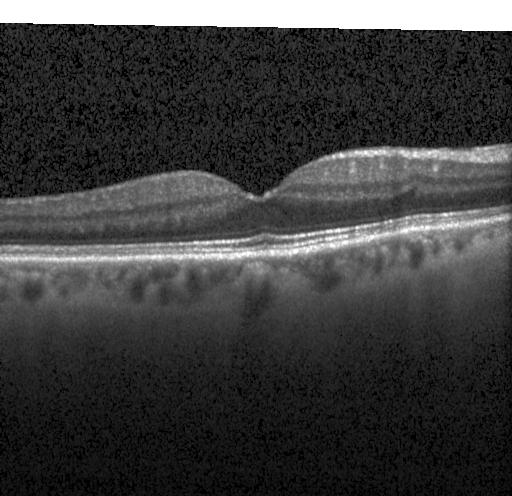
Heidelberg Spectralis; optical coherence tomography B-scan; centered on the fovea; spectral-domain optical coherence tomography
Diagnosis: no CNV, no DME, and no drusen.